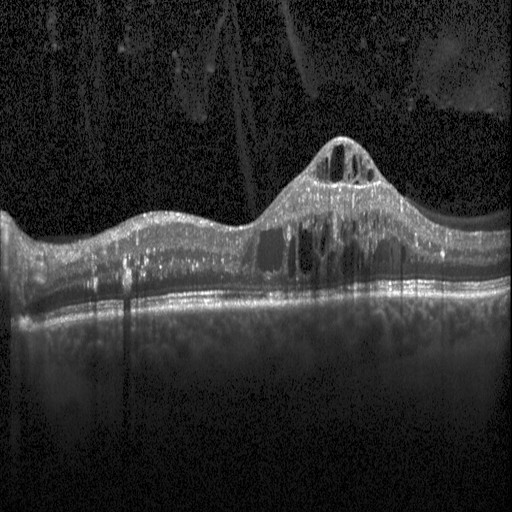 Assessment: DME.